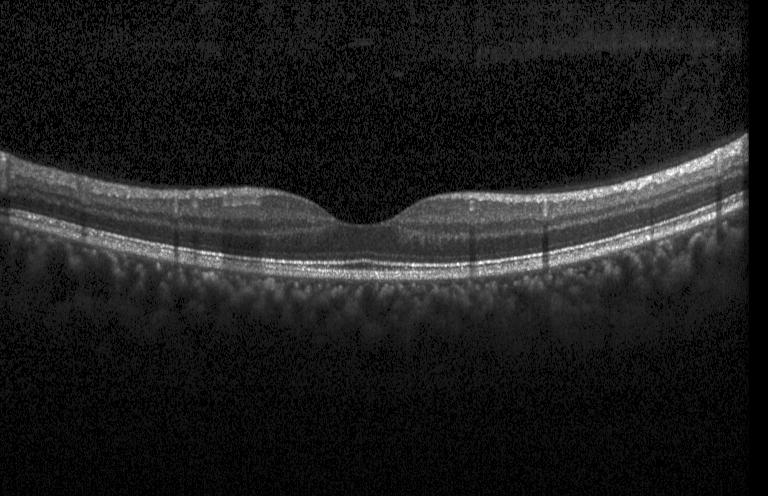
Finding: neither CNV, DME, nor drusen.